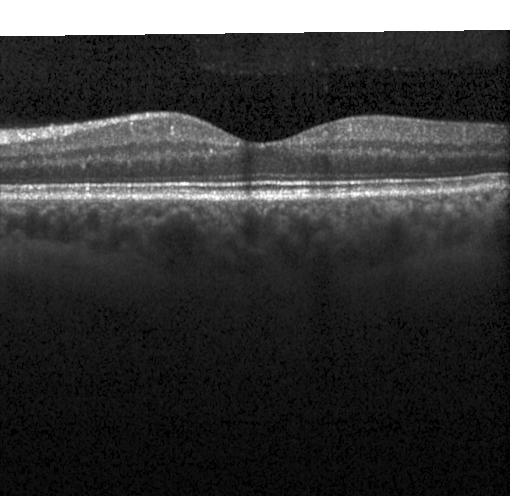

Optical coherence tomography B-scan
Diagnosis: no evidence of choroidal neovascularization, diabetic macular edema, or drusen.